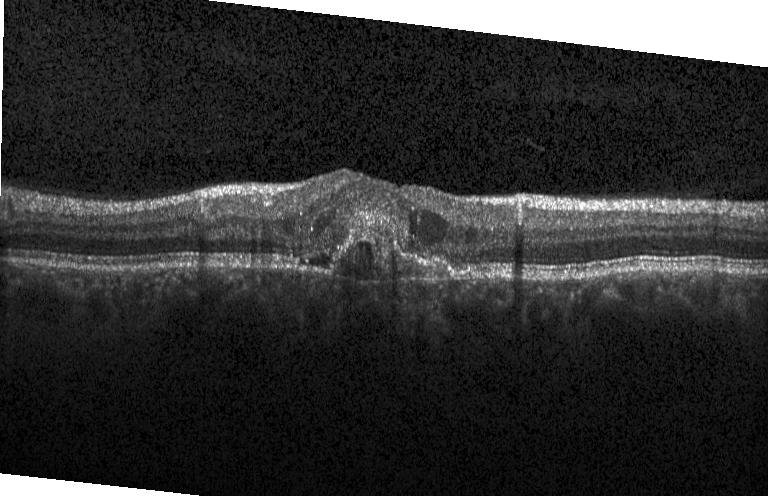
Macular OCT demonstrating CNV.